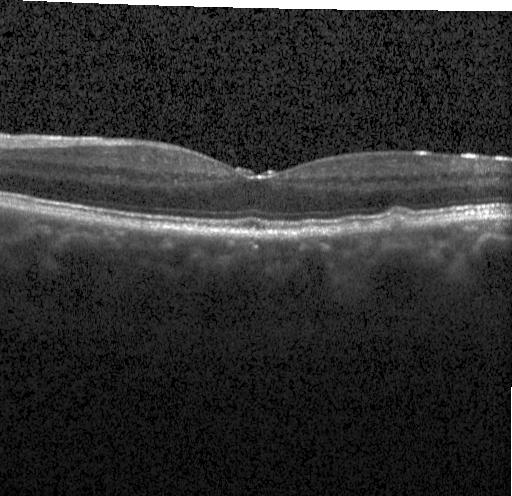

Retinal OCT cross-section — This B-scan demonstrates sub-RPE drusenoid deposits.